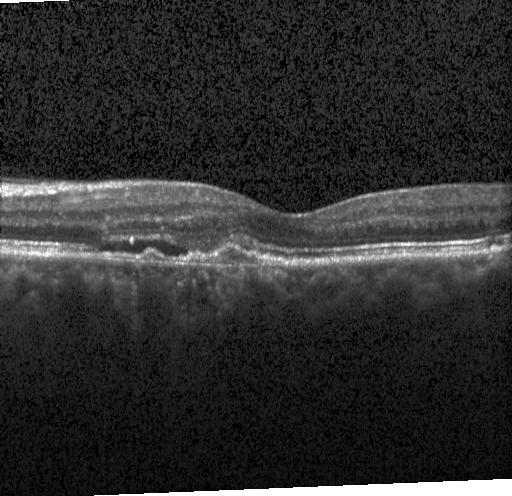 Impression: choroidal neovascularization.